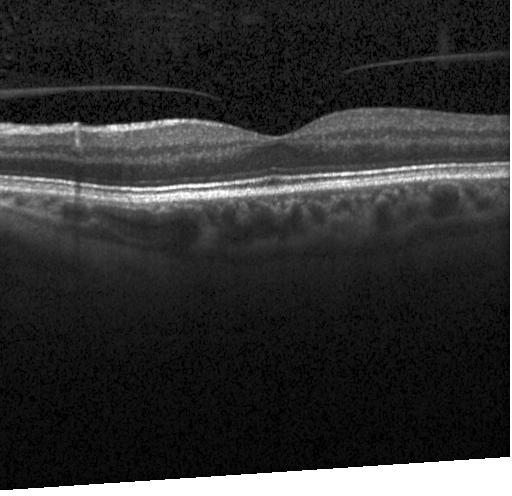

Retinal OCT cross-section. Fovea-centered. Heidelberg Spectralis OCT system
Assessment: no evidence of choroidal neovascularization, diabetic macular edema, or drusen.